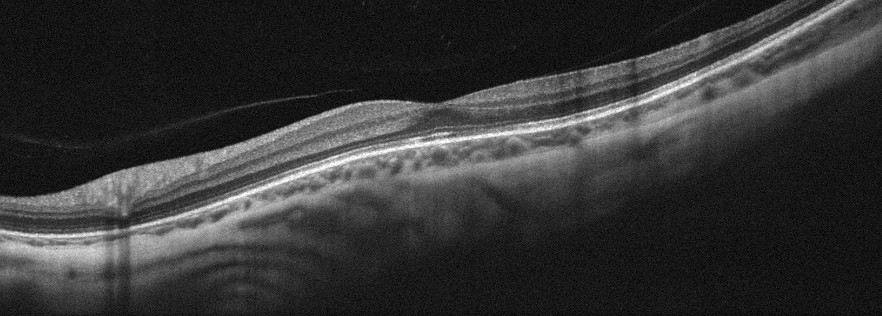 Finding: no evidence of AMD, DME, ERM, RAO, RVO, or VID.